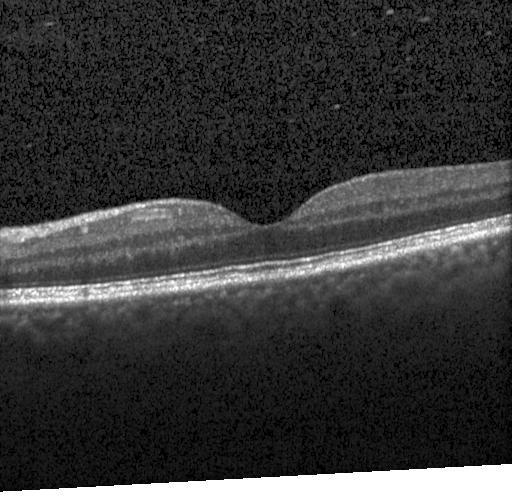
Retinal OCT cross-section; SD-OCT; Heidelberg Spectralis OCT system. Finding: no choroidal neovascularization, diabetic macular edema, or drusen.